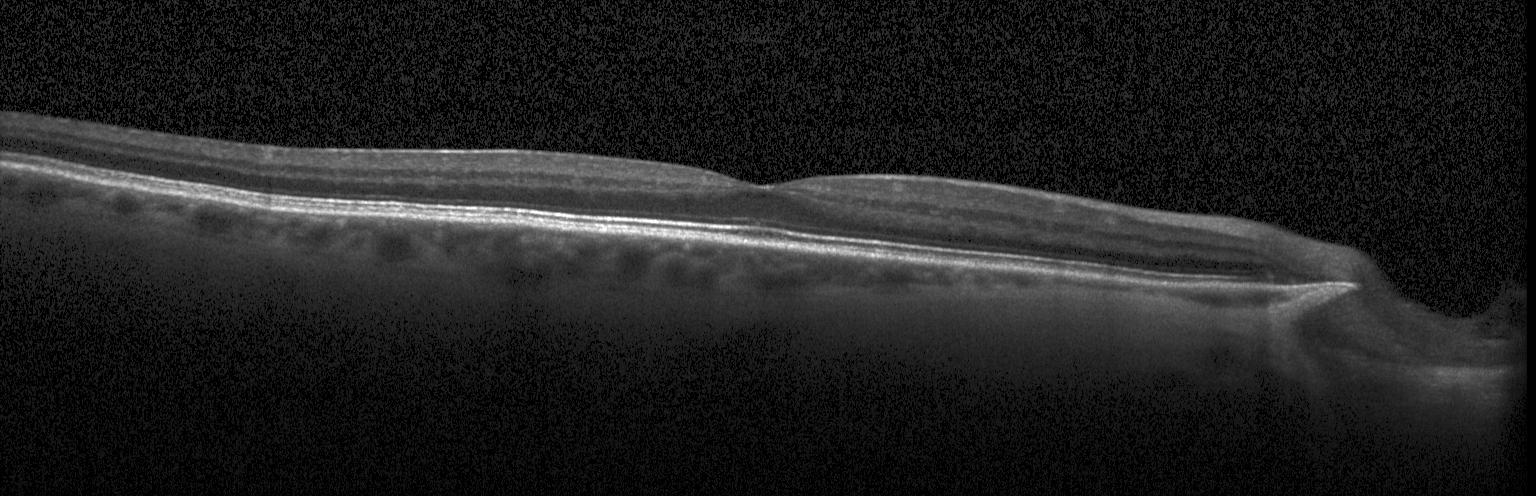
Centered on the fovea; retinal OCT B-scan; spectral-domain optical coherence tomography.
OCT finding: neither CNV, DME, nor drusen.